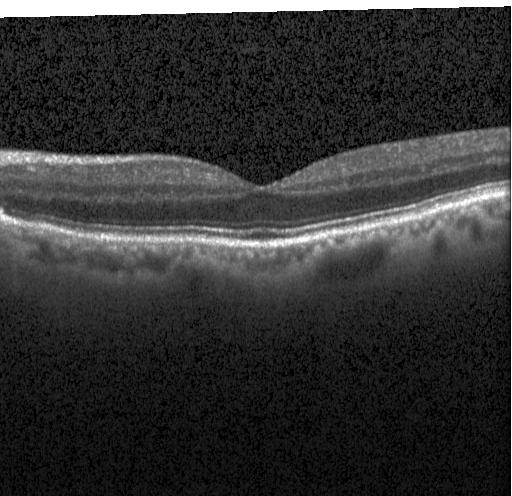
OCT line scan, fovea-centered, Heidelberg Spectralis — Neither CNV, DME, nor drusen.